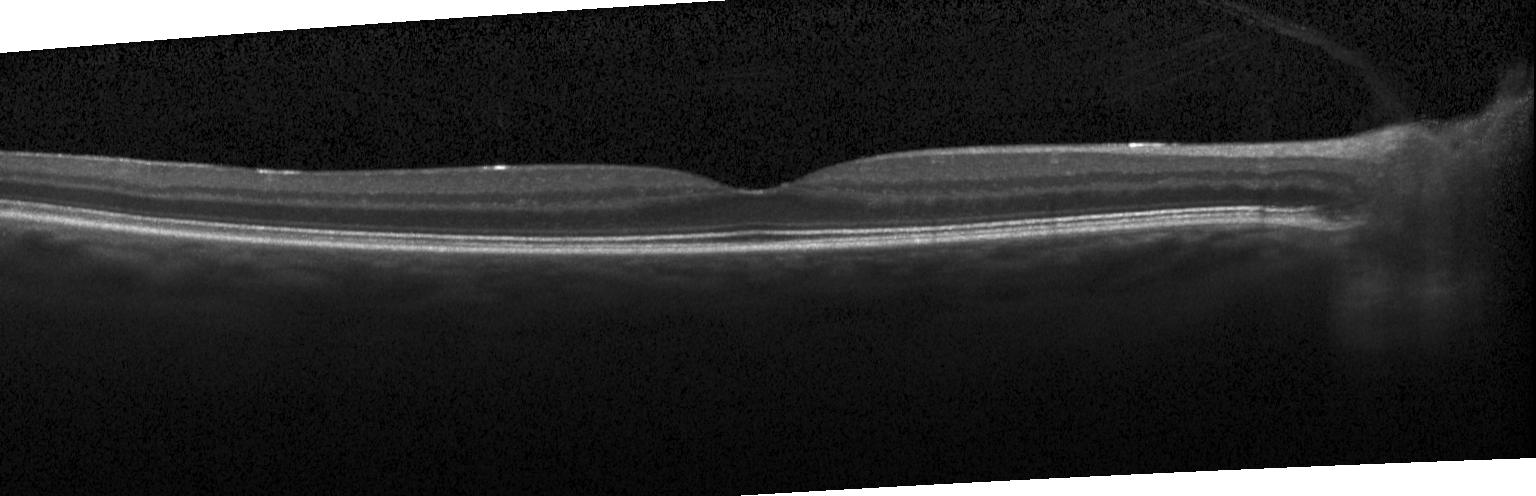 OCT scan showing no choroidal neovascularization, diabetic macular edema, or drusen.